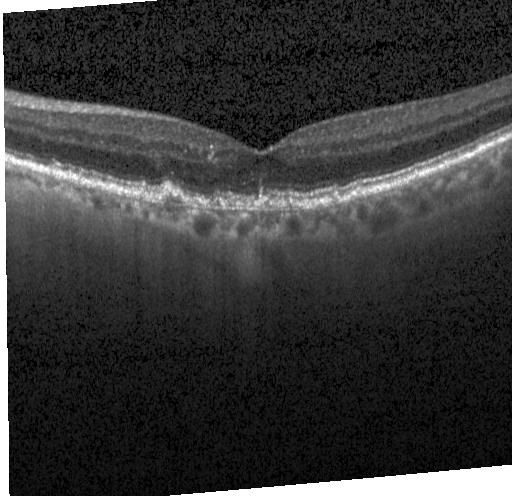

OCT B-scan showing drusen.